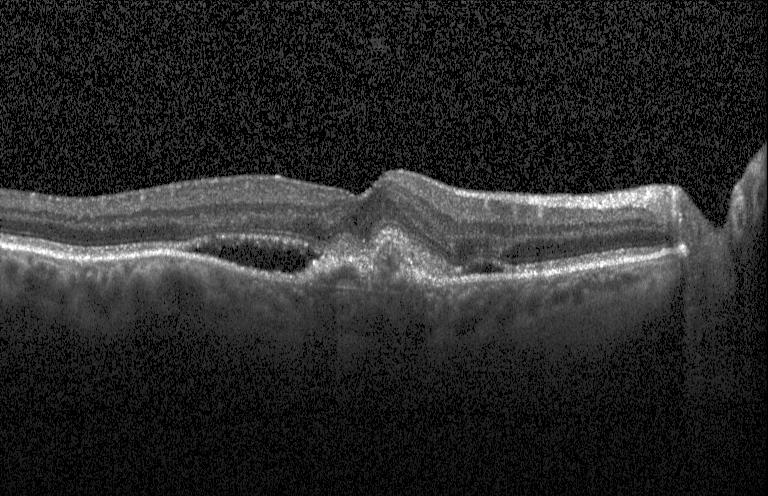

OCT B-scan. The scan shows a choroidal neovascular membrane.